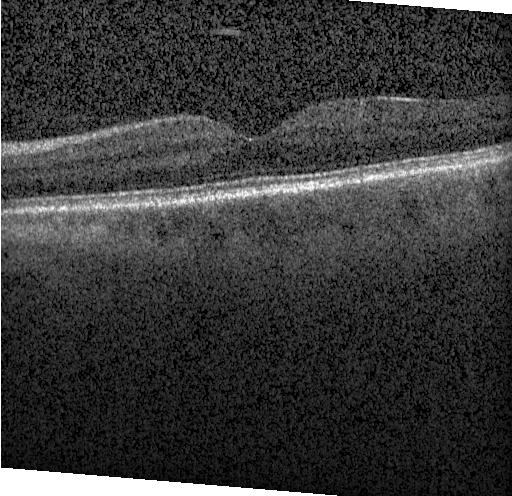
OCT finding: no choroidal neovascularization, no diabetic macular edema, and no drusen.